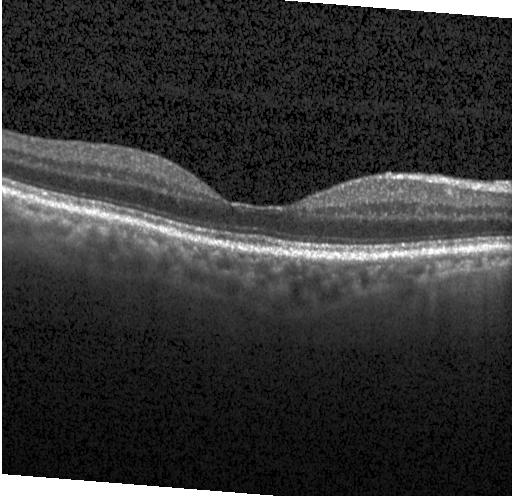 Optical coherence tomography B-scan. Neither choroidal neovascularization, diabetic macular edema, nor drusen.